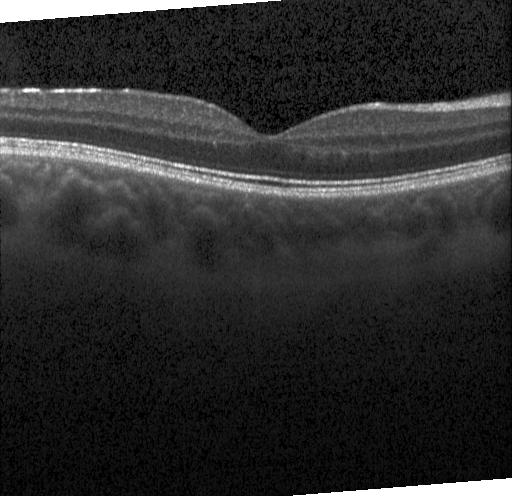
Optical coherence tomography B-scan, SD-OCT, centered on the fovea — No choroidal neovascularization, no diabetic macular edema, and no drusen.